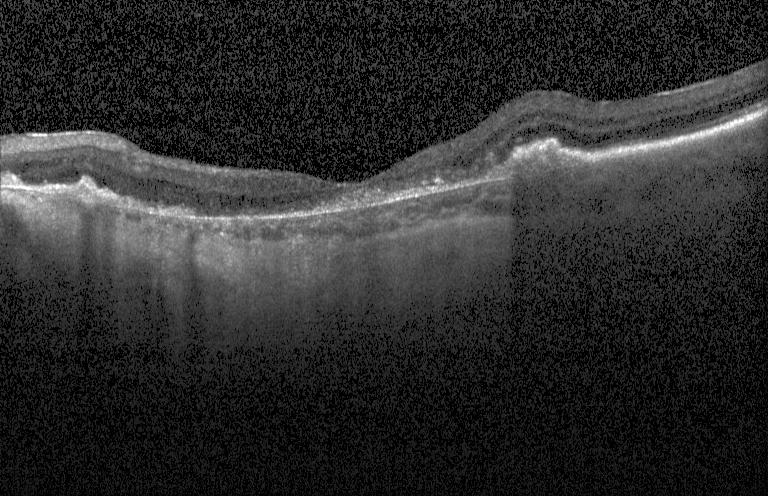 This B-scan demonstrates a choroidal neovascular membrane.